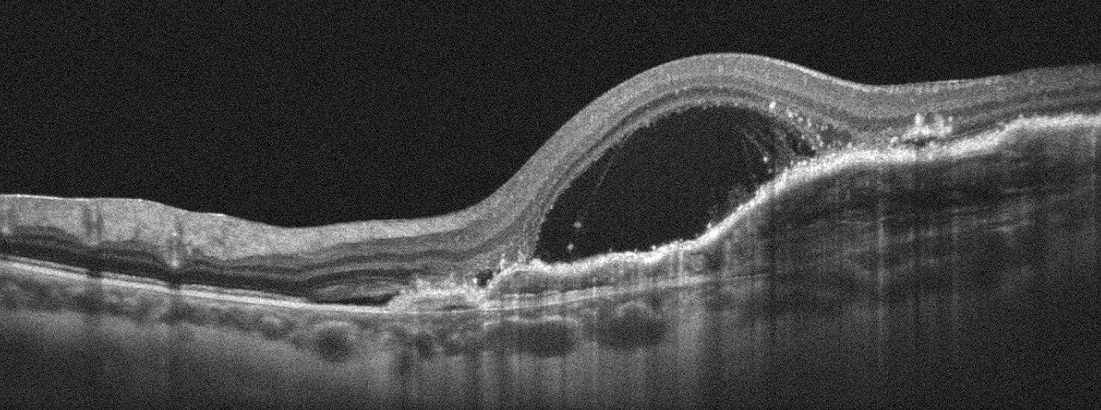

OCT B-scan — Finding: age-related macular degeneration (AMD).